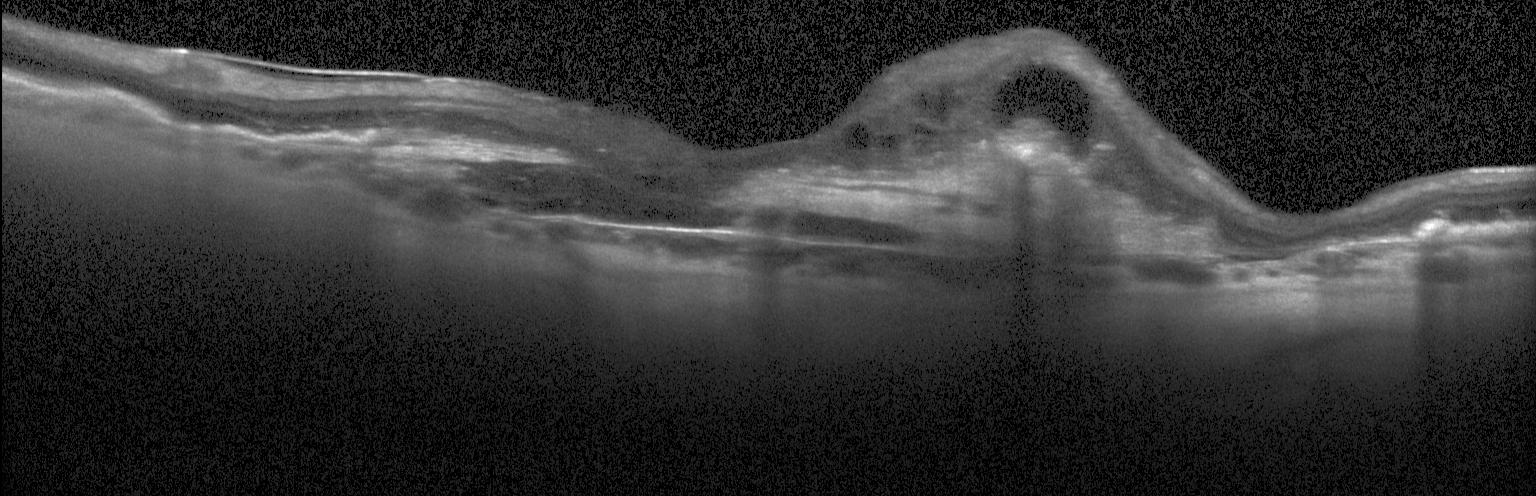 Retinal OCT cross-section
Diagnosis: CNV.